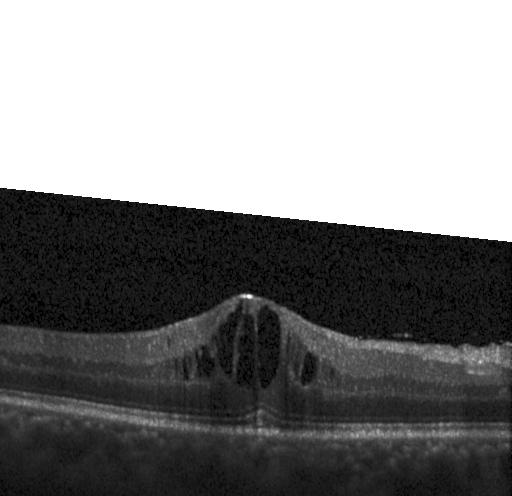

OCT line scan.
Finding: diabetic macular edema (DME).